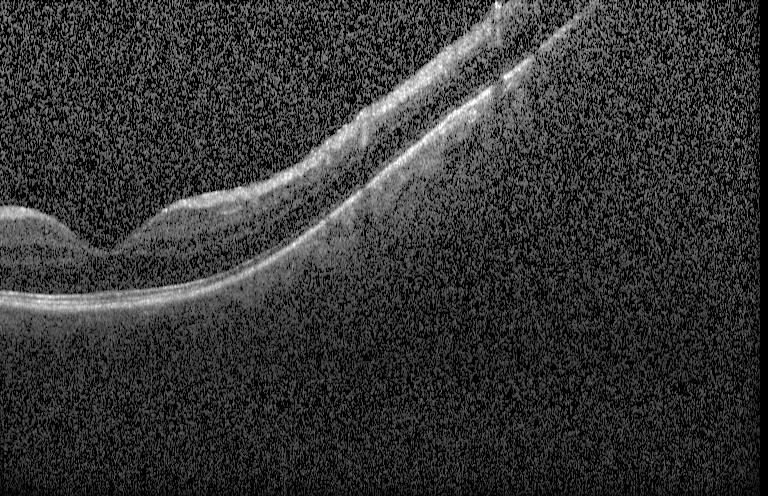

Optical coherence tomography scan. Through the macula.
Diagnosis: neither choroidal neovascularization, diabetic macular edema, nor drusen.